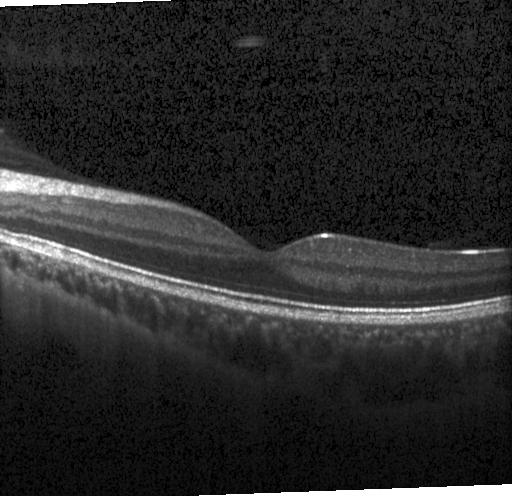

Through the macula; spectral-domain optical coherence tomography; acquired on a Heidelberg Spectralis; optical coherence tomography scan.
Macular OCT: neither choroidal neovascularization, diabetic macular edema, nor drusen.